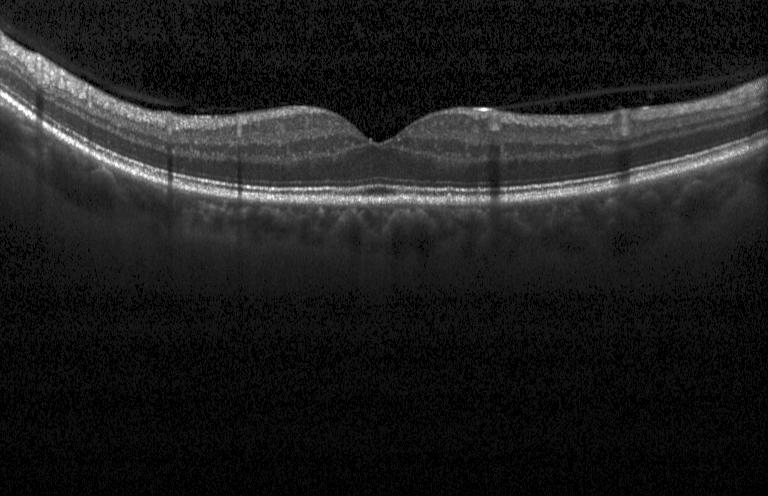
Spectral-domain optical coherence tomography. OCT B-scan. This B-scan demonstrates no choroidal neovascularization, no diabetic macular edema, and no drusen.